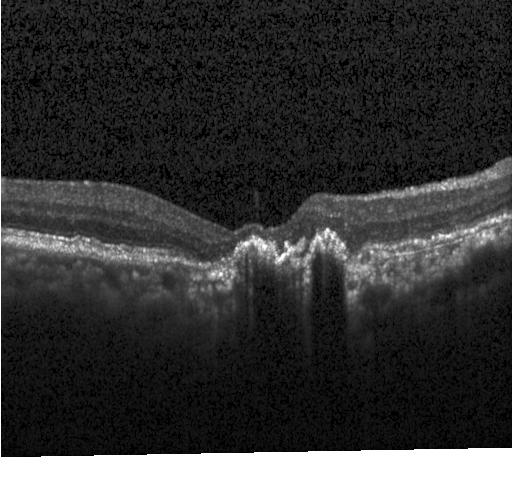
Instrument: Heidelberg Spectralis; retinal OCT B-scan; centered on the fovea; spectral-domain OCT — Assessment: a choroidal neovascular membrane.